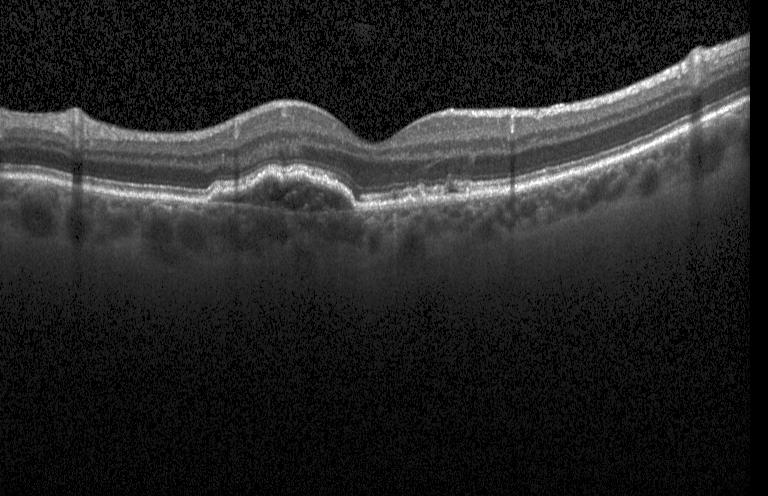 Centered on the fovea. Optical coherence tomography scan — Impression: choroidal neovascularization (CNV).